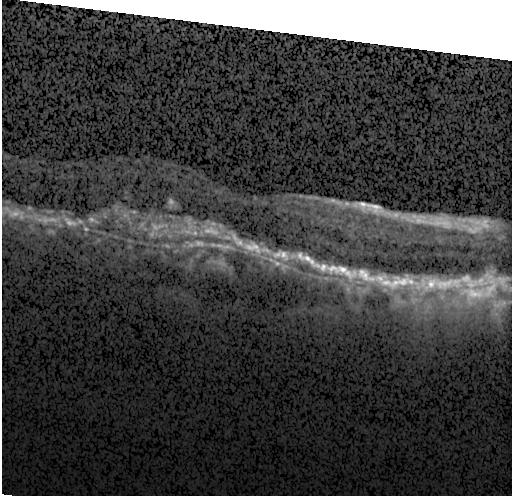 Spectral-domain optical coherence tomography. Optical coherence tomography B-scan. Instrument: Heidelberg Spectralis. Horizontal scan through the fovea. Macular OCT: choroidal neovascularization (CNV).